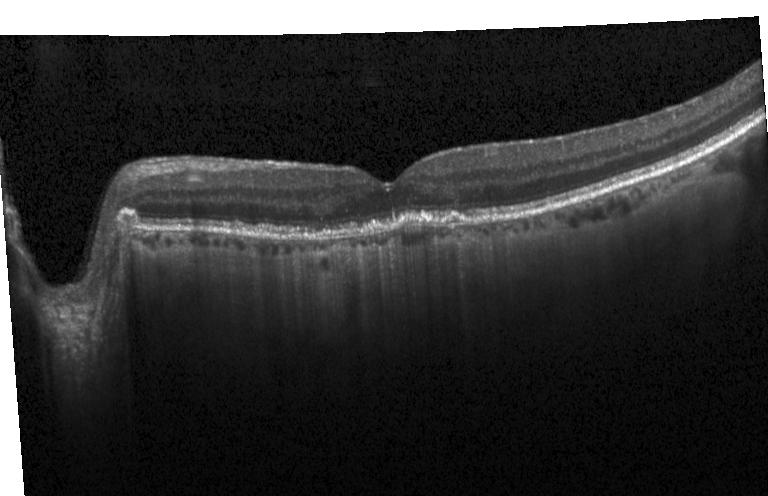
OCT scan showing drusen.